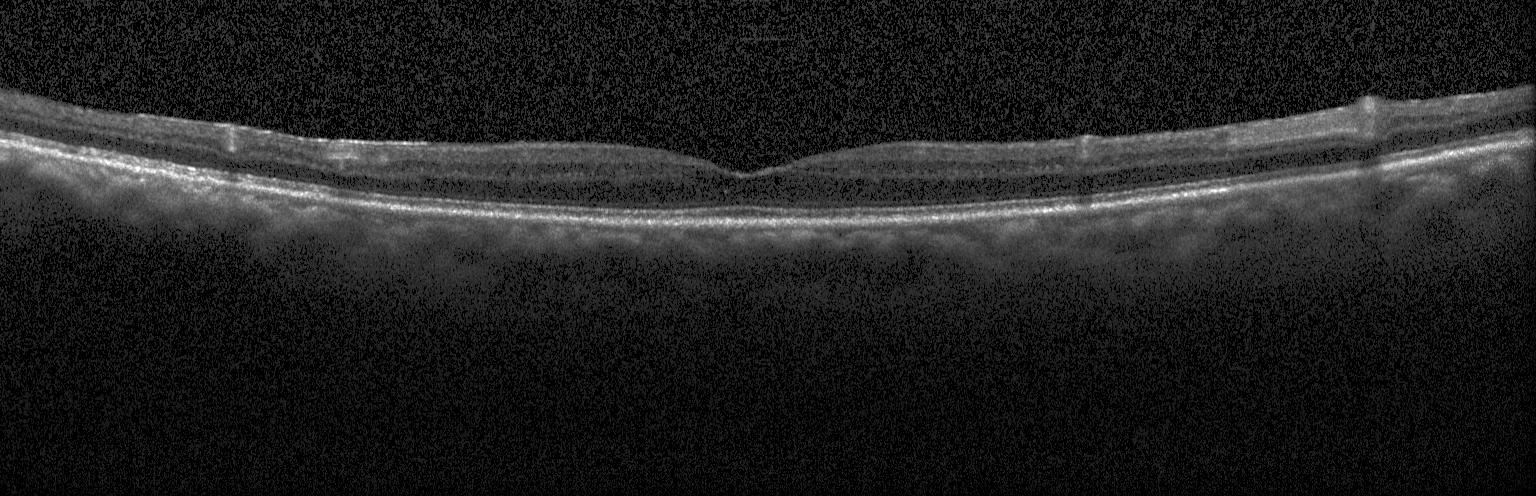

Optical coherence tomography scan. Impression: no evidence of CNV, DME, or drusen.